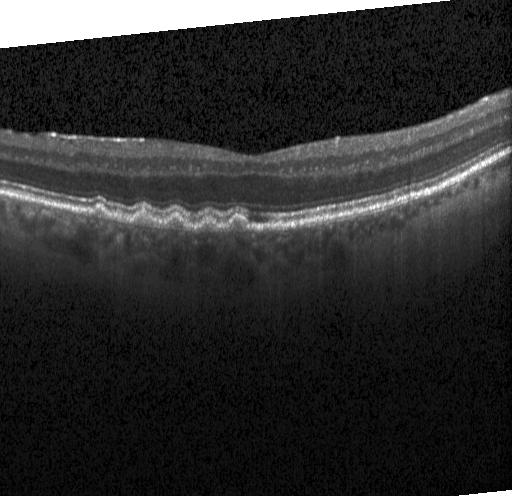 Finding: drusen.